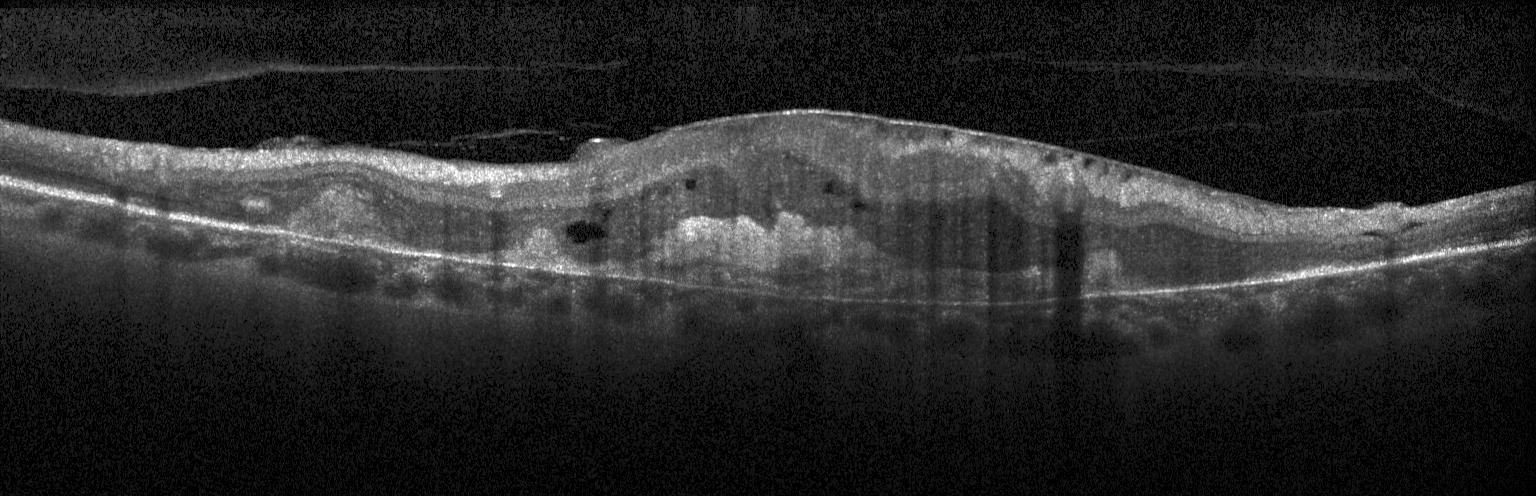 Impression: a choroidal neovascular membrane.